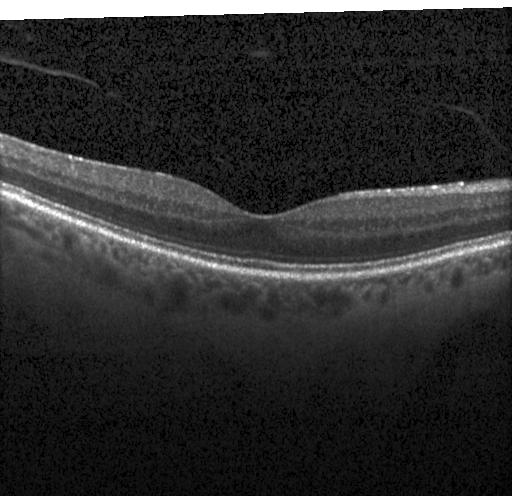 Instrument: Heidelberg Spectralis; spectral-domain OCT; horizontal scan through the fovea; OCT B-scan — Impression: no choroidal neovascularization, no diabetic macular edema, and no drusen.